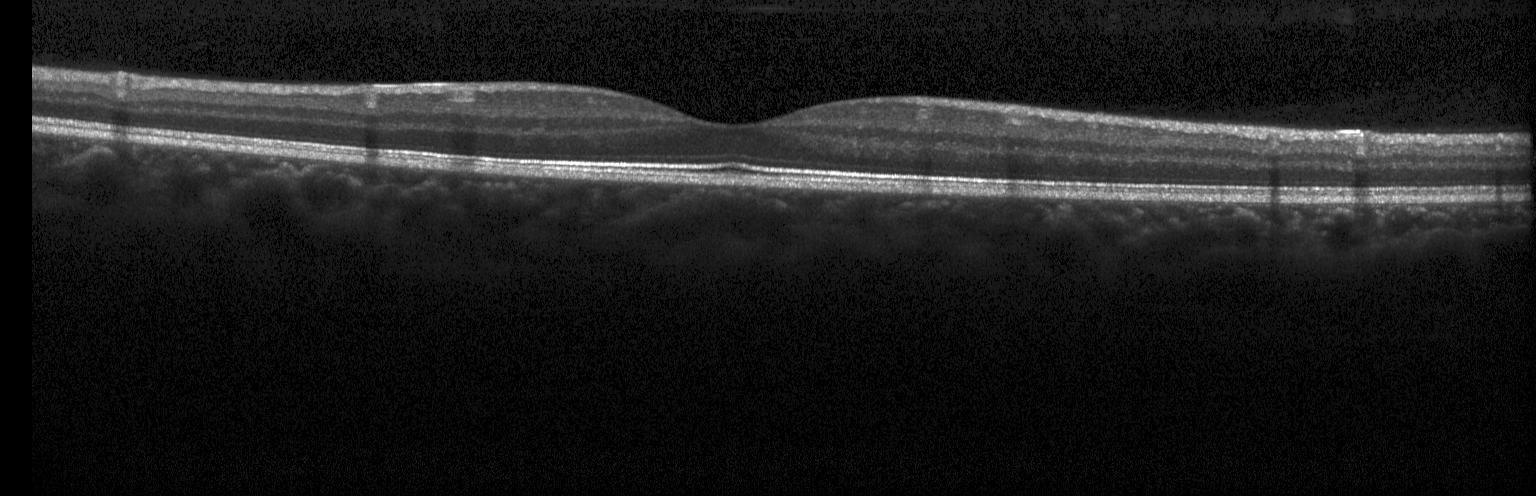 OCT B-scan — Finding: no CNV, no DME, and no drusen.